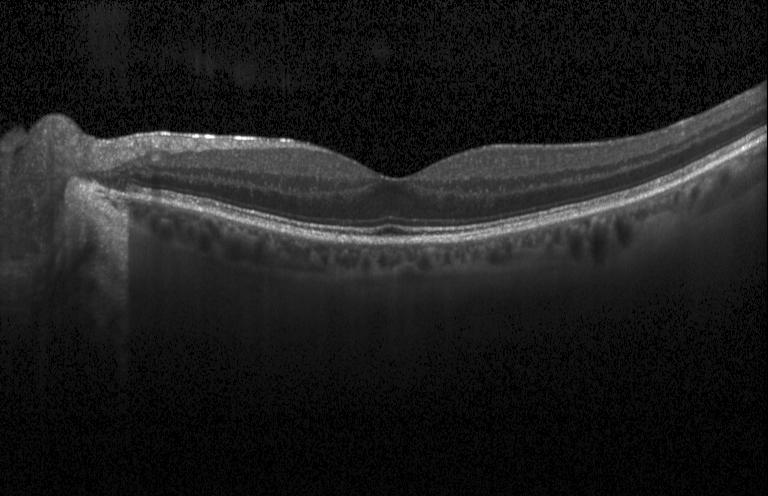

OCT finding: no choroidal neovascularization, no diabetic macular edema, and no drusen.